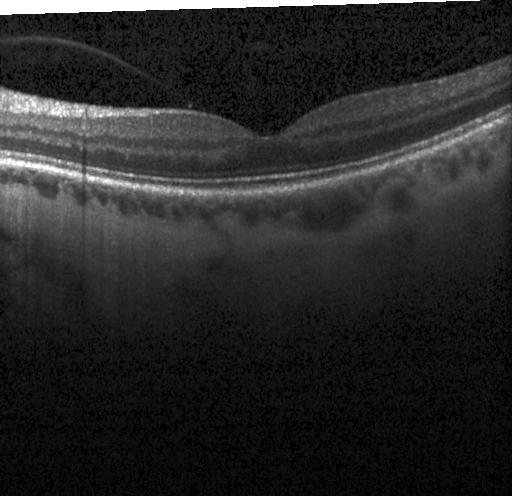
Through the macula · spectral-domain OCT · instrument: Heidelberg Spectralis · retinal OCT B-scan — The scan shows no choroidal neovascularization, diabetic macular edema, or drusen.